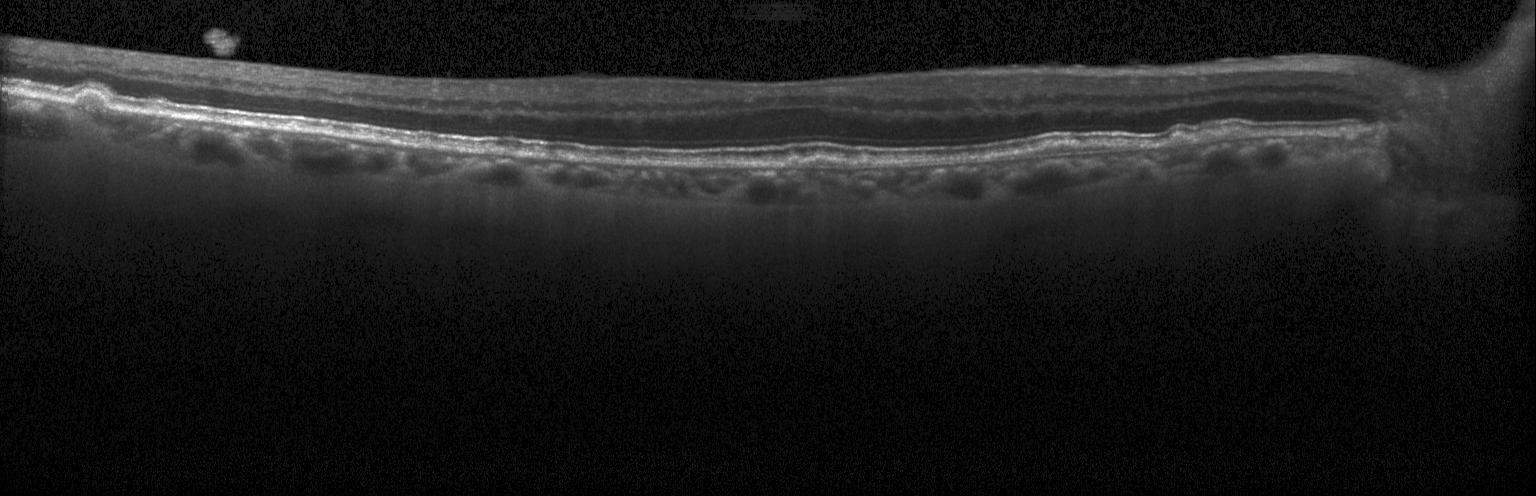

Through the macula. OCT B-scan. Instrument: Heidelberg Spectralis. Spectral-domain OCT.
Assessment: drusen.